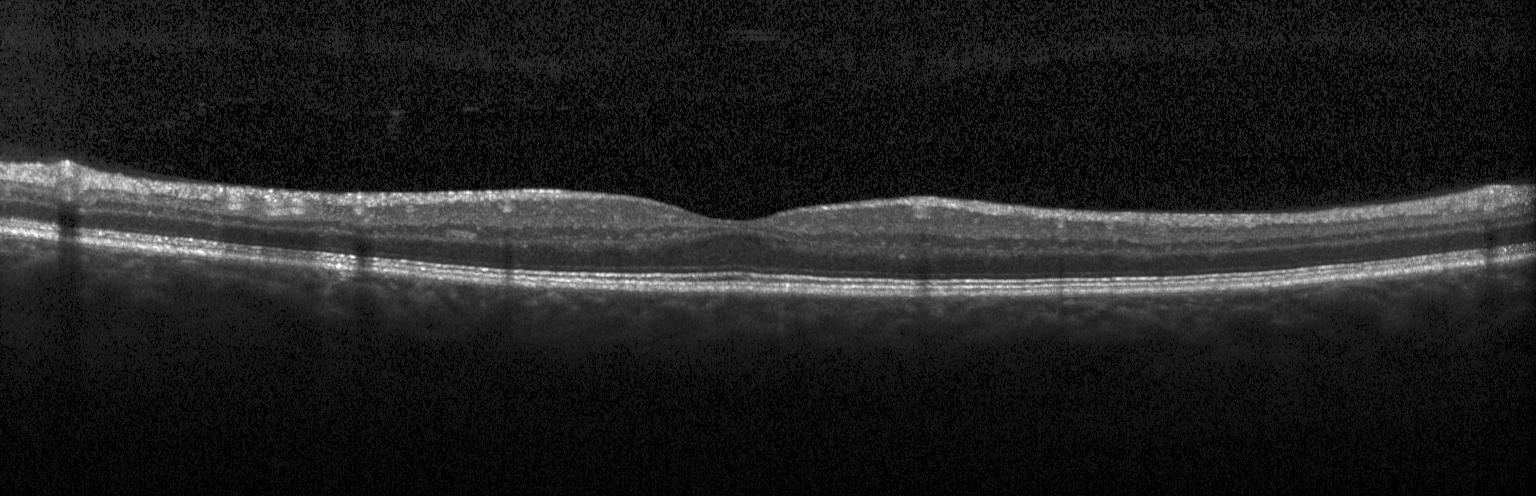 Macular OCT demonstrating no evidence of choroidal neovascularization, diabetic macular edema, or drusen.